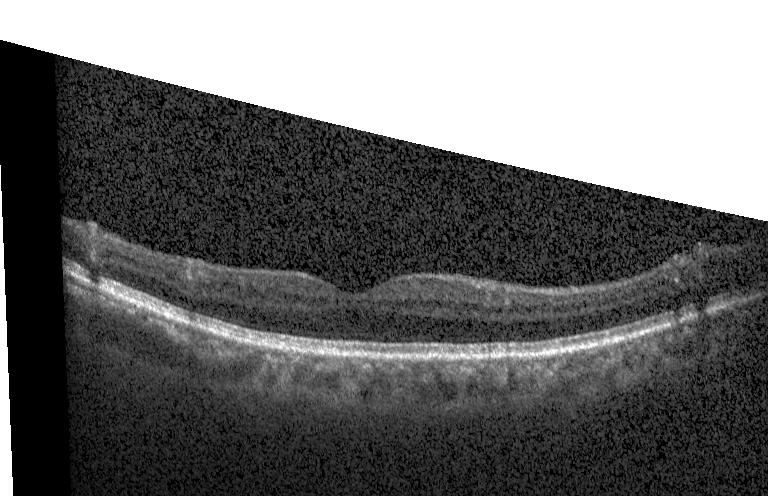

Retinal OCT cross-section, through the macula, SD-OCT — Macular OCT: neither choroidal neovascularization, diabetic macular edema, nor drusen.